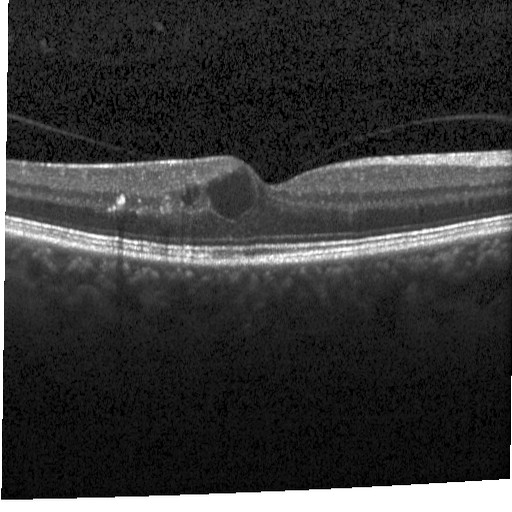

Spectral-domain OCT B-scan: DME.